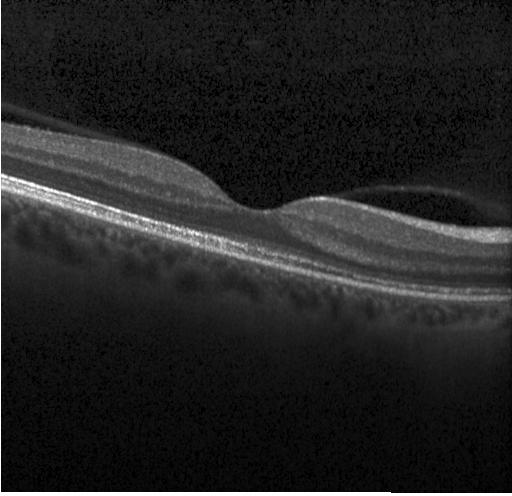 Retinal OCT cross-section showing no evidence of choroidal neovascularization, diabetic macular edema, or drusen.